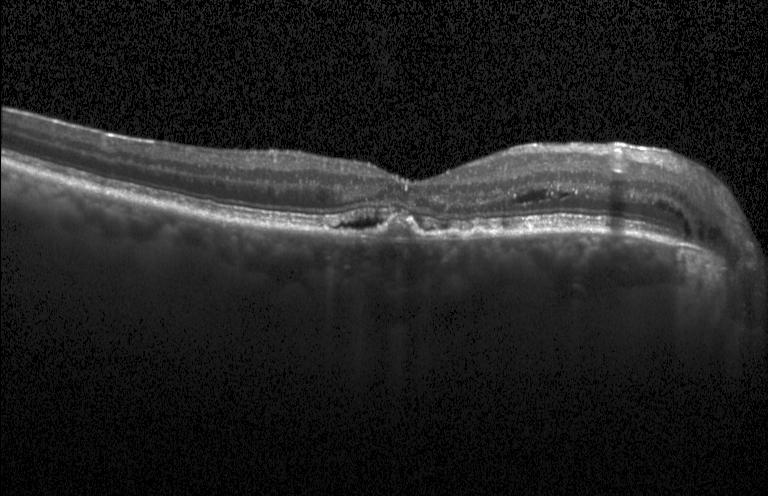
SD-OCT · optical coherence tomography B-scan · instrument: Heidelberg Spectralis · centered on the fovea. Diagnosis: a choroidal neovascular membrane.